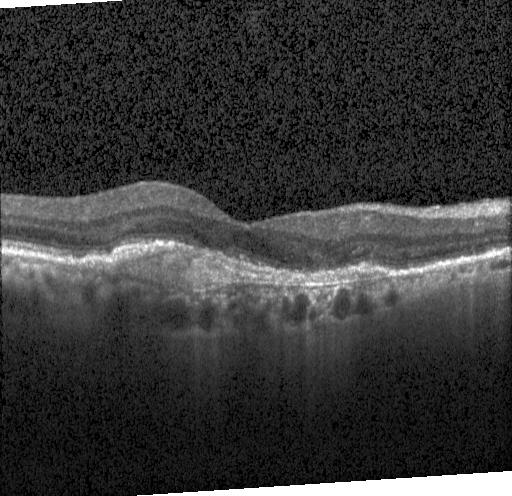 Impression: CNV.